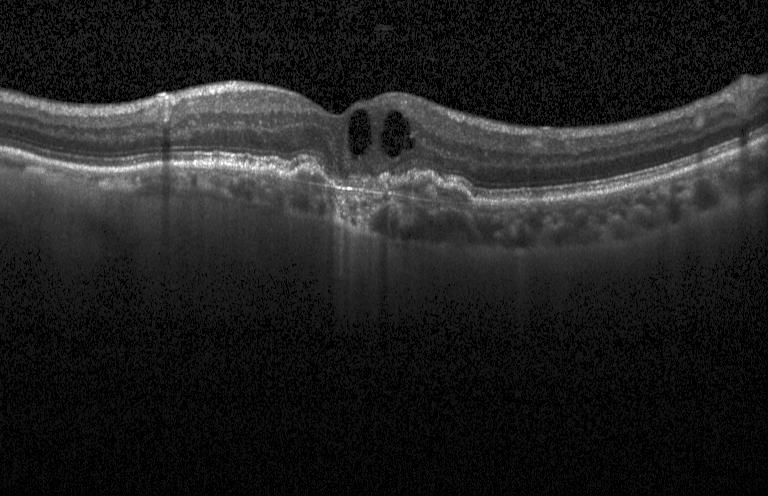
Optical coherence tomography B-scan, through the macula, spectral-domain OCT, Heidelberg Spectralis
Diagnosis: choroidal neovascularization.